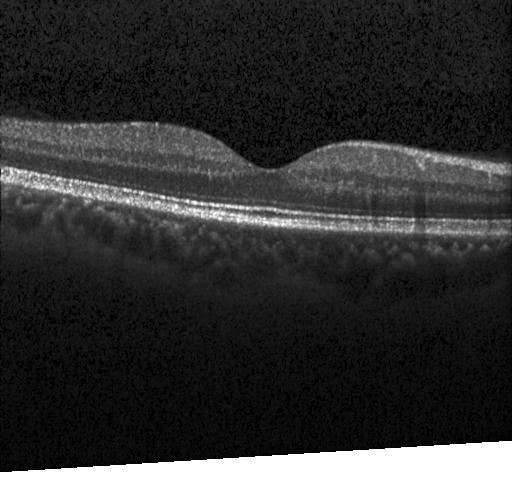 Retinal OCT cross-section, instrument: Heidelberg Spectralis, spectral-domain OCT.
Macular OCT: no evidence of CNV, DME, or drusen.